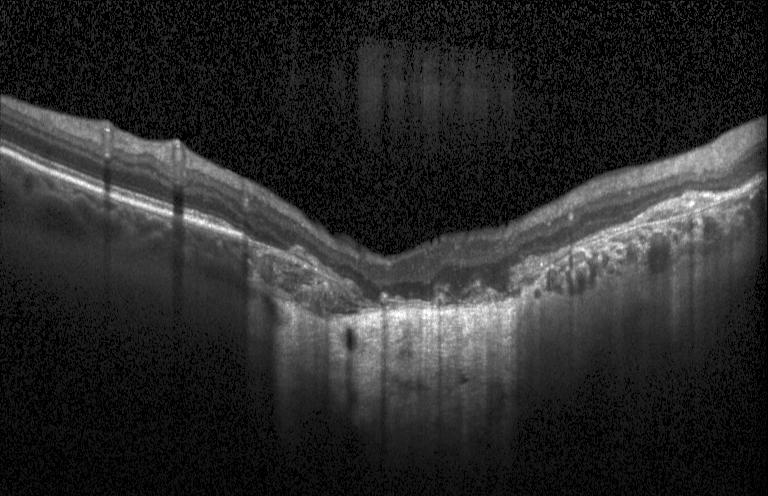
Assessment: a choroidal neovascular membrane.